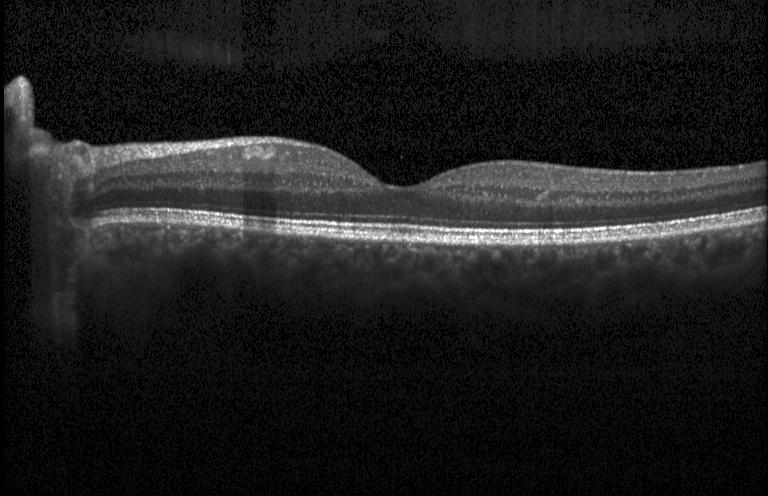 No evidence of CNV, DME, or drusen.